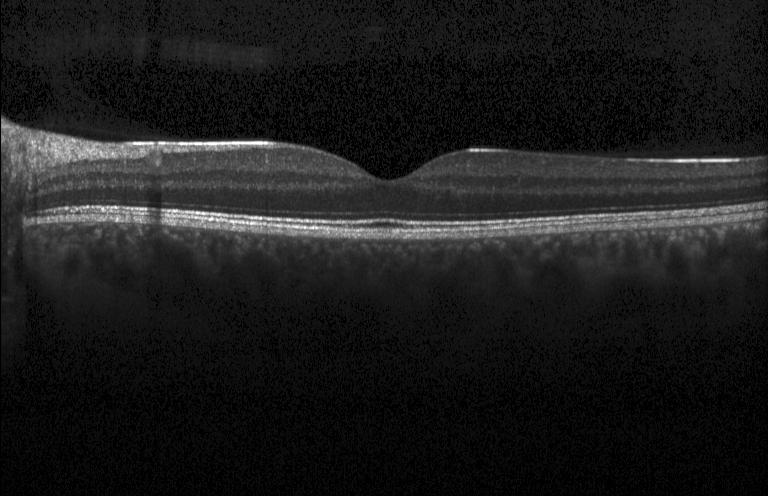

Retinal OCT B-scan · instrument: Heidelberg Spectralis. Assessment: no CNV, no DME, and no drusen.